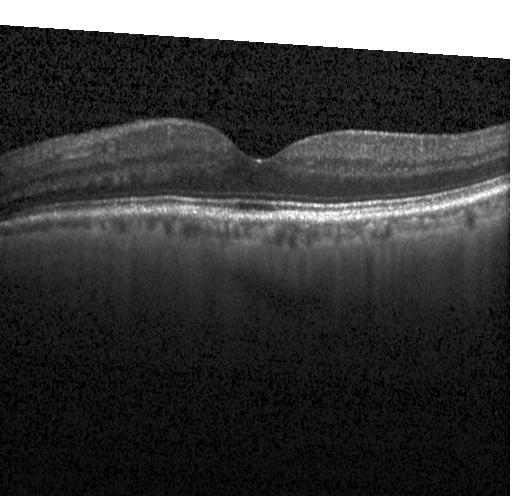
Retinal OCT B-scan. Spectral-domain OCT. Centered on the fovea. Acquired on a Heidelberg Spectralis — Neither choroidal neovascularization, diabetic macular edema, nor drusen.